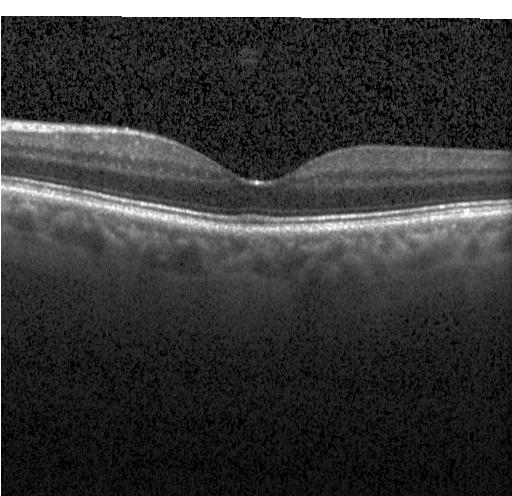
Optical coherence tomography B-scan — Impression: no evidence of choroidal neovascularization, diabetic macular edema, or drusen.